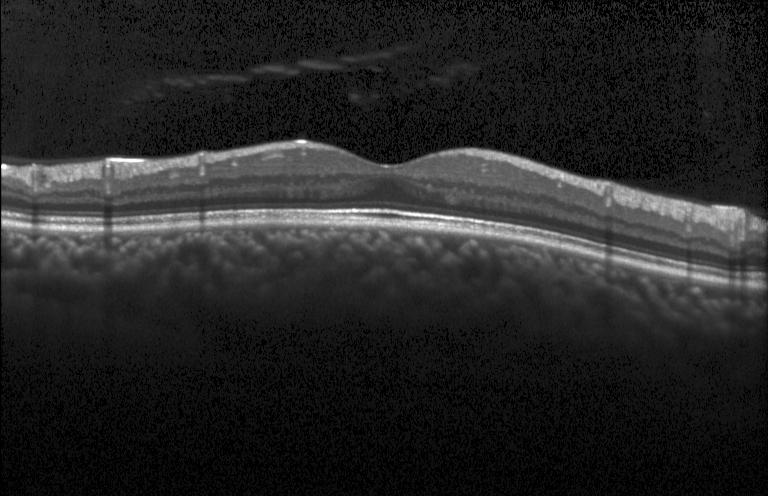
OCT B-scan showing no evidence of choroidal neovascularization, diabetic macular edema, or drusen.